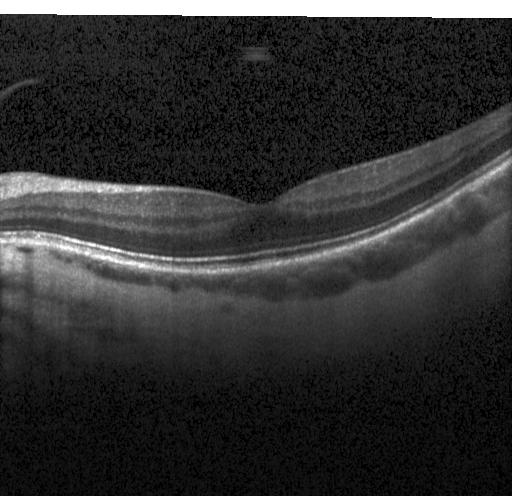
The scan shows neither choroidal neovascularization, diabetic macular edema, nor drusen.